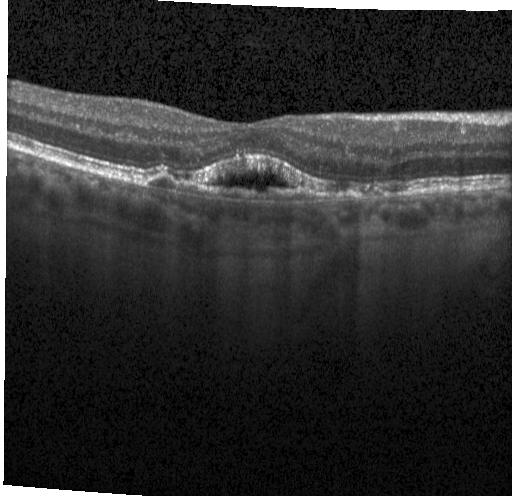

Dx: a choroidal neovascular membrane.